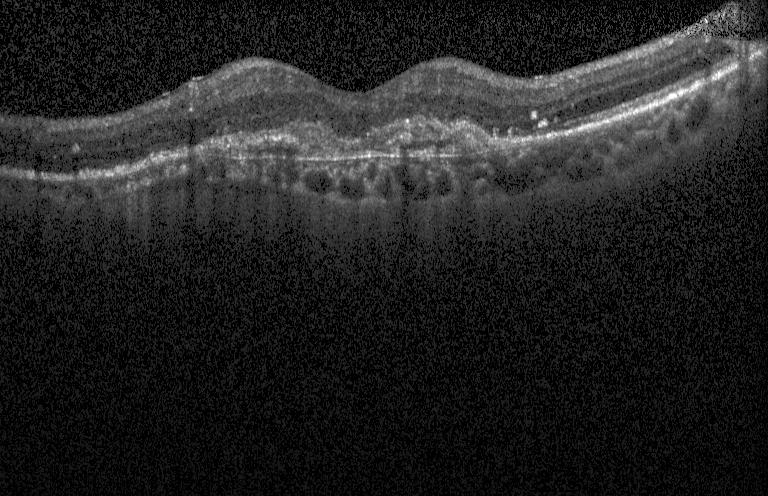
Impression: a choroidal neovascular membrane.